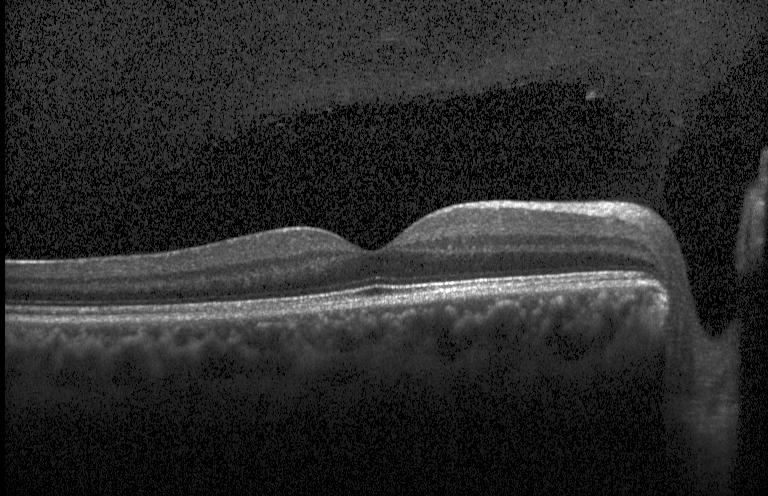 SD-OCT · optical coherence tomography scan — Finding: neither choroidal neovascularization, diabetic macular edema, nor drusen.